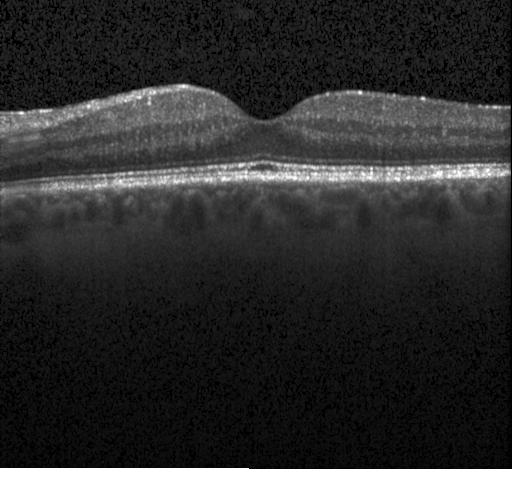
Retinal OCT cross-section showing no CNV, DME, or drusen.